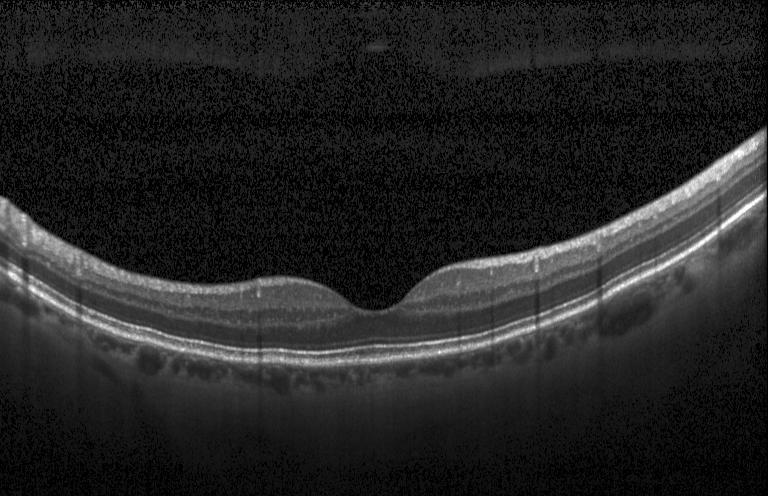
Macular OCT: no choroidal neovascularization, no diabetic macular edema, and no drusen.